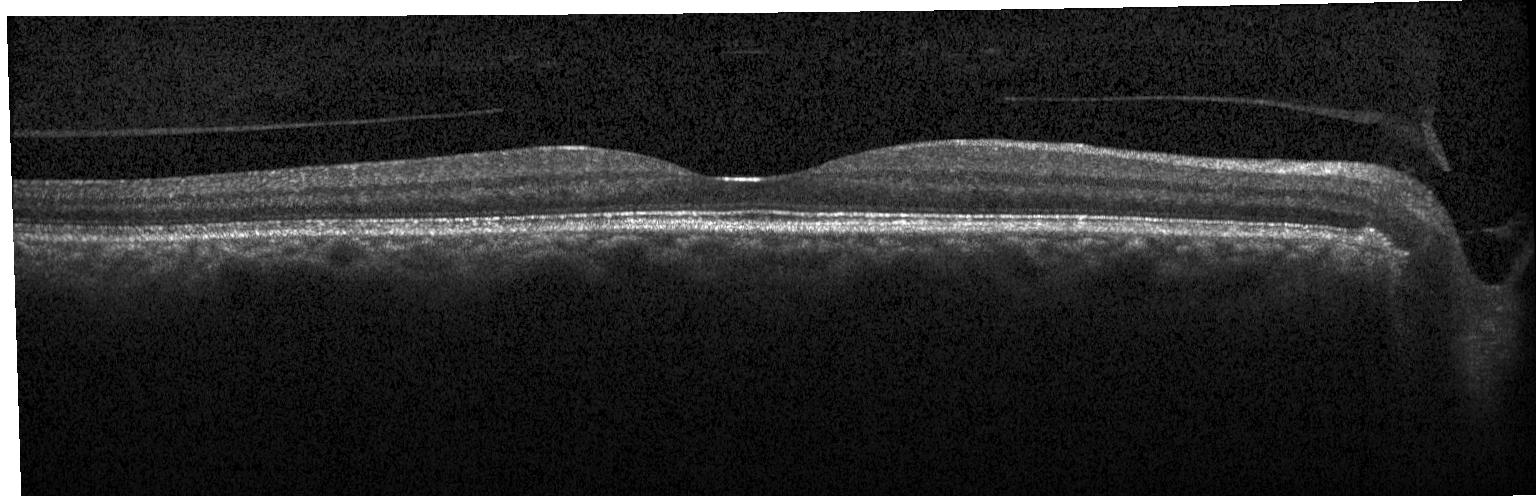
Retinal OCT cross-section. Impression: neither choroidal neovascularization, diabetic macular edema, nor drusen.